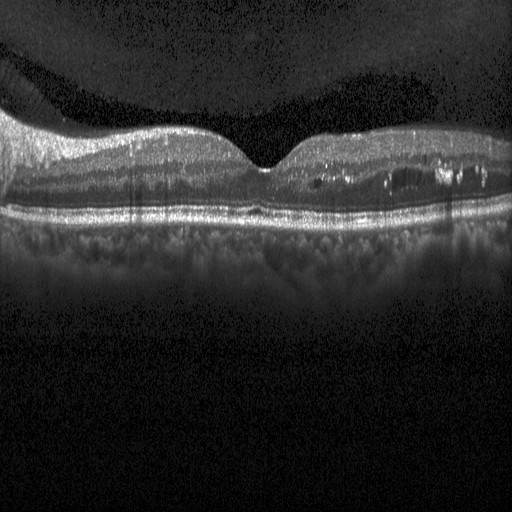

Optical coherence tomography scan. Instrument: Heidelberg Spectralis
Diagnosis: diabetic macular edema (DME).